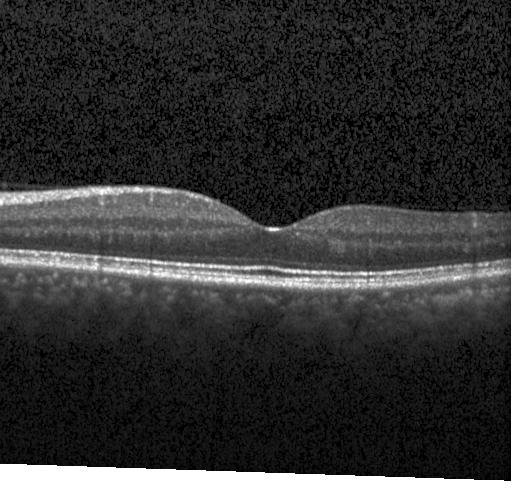

No evidence of choroidal neovascularization, diabetic macular edema, or drusen.